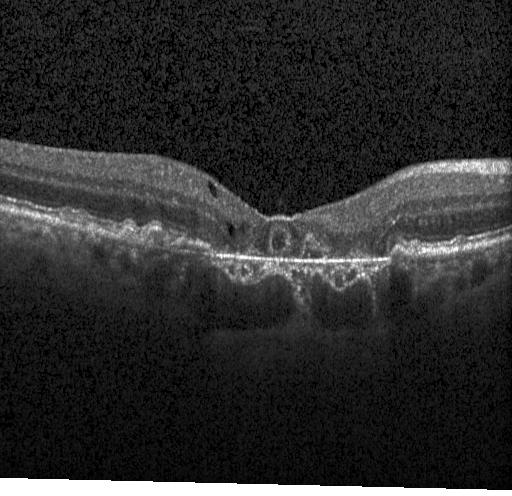

This B-scan demonstrates a choroidal neovascular membrane.